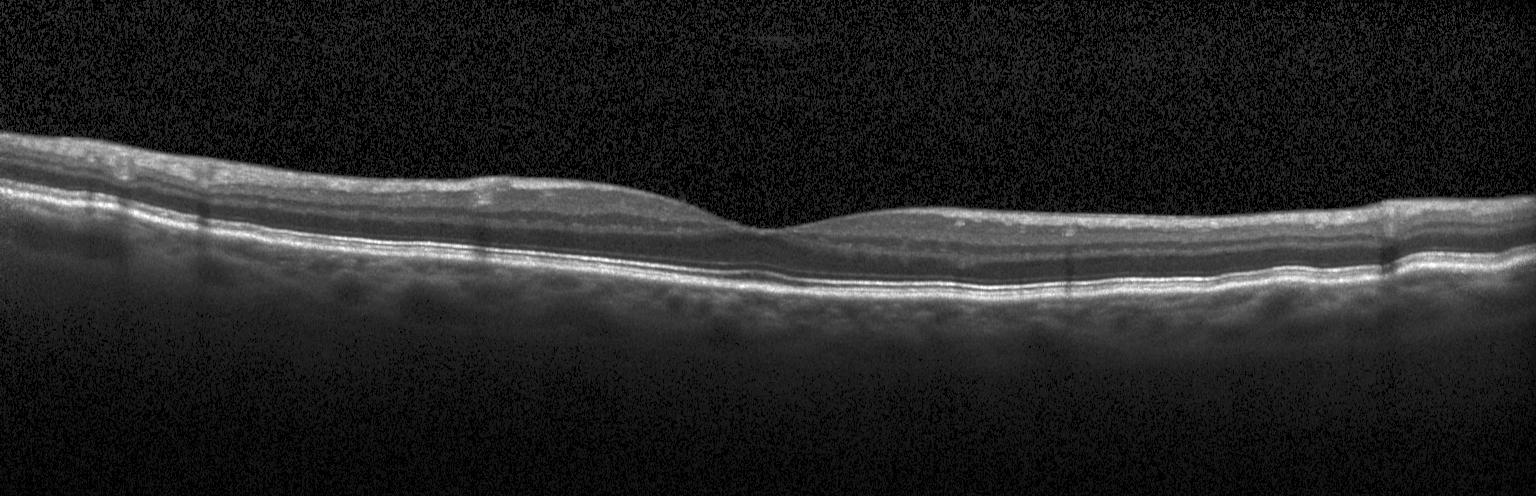

Macular OCT: no evidence of choroidal neovascularization, diabetic macular edema, or drusen.